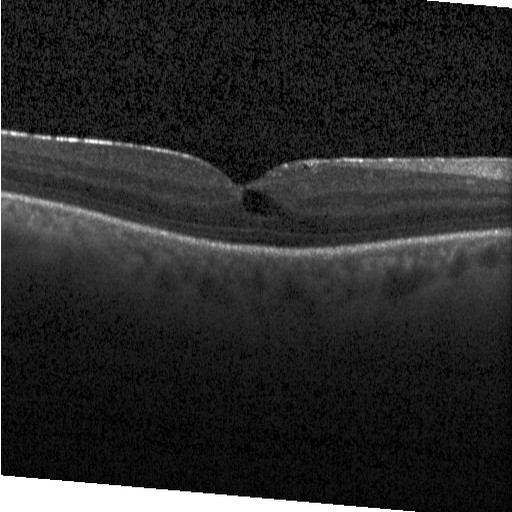
SD-OCT, optical coherence tomography B-scan, instrument: Heidelberg Spectralis. DME.